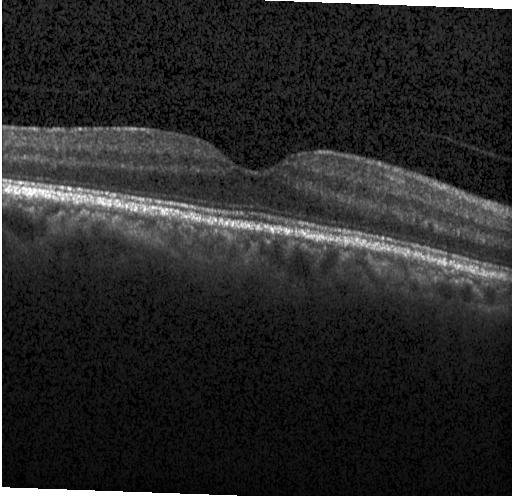 Diagnosis: neither choroidal neovascularization, diabetic macular edema, nor drusen.